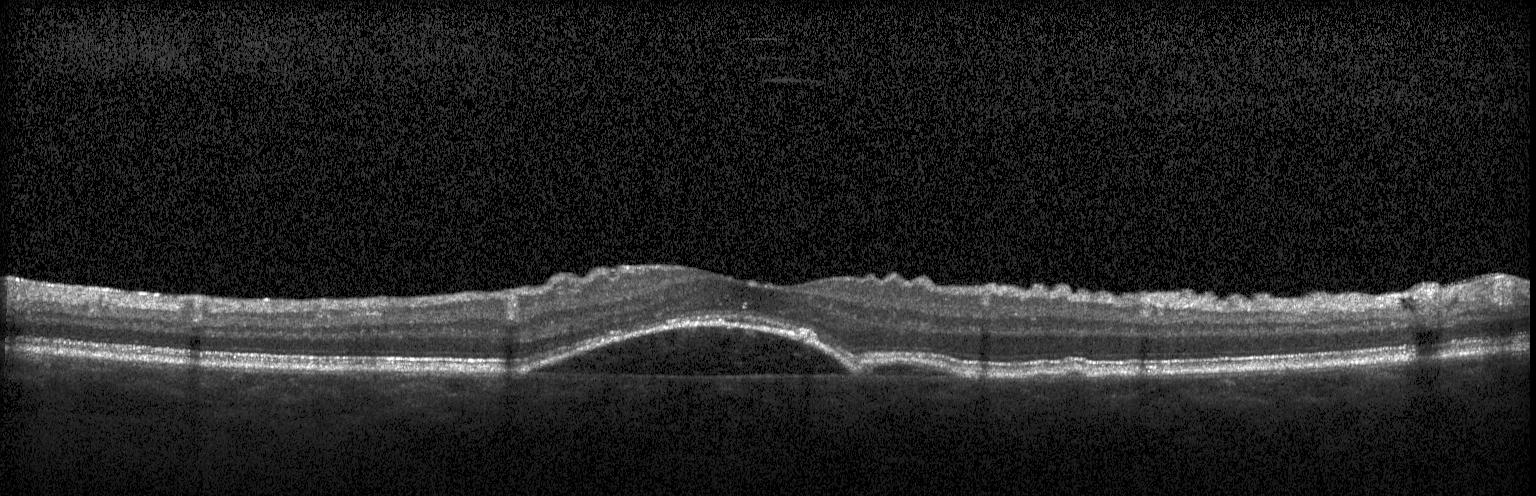

Diagnosis: a choroidal neovascular membrane.